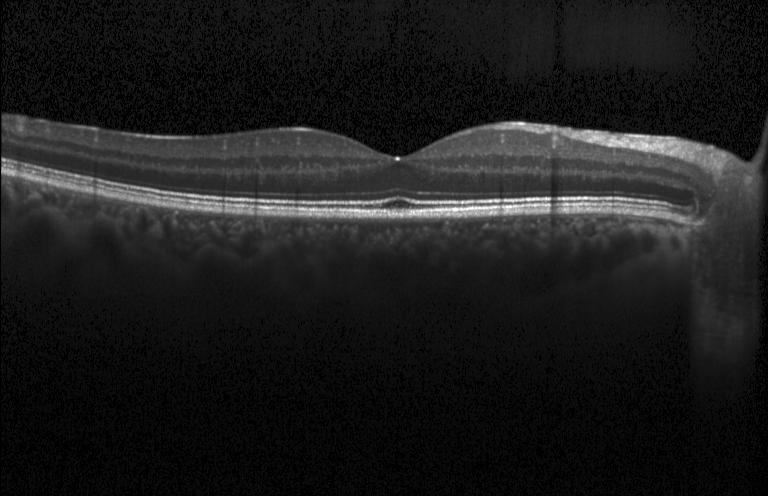 Instrument: Heidelberg Spectralis; fovea-centered; OCT line scan; SD-OCT.
The scan shows no choroidal neovascularization, diabetic macular edema, or drusen.